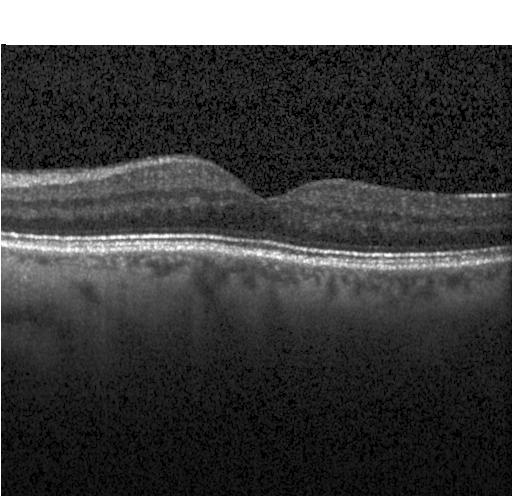 OCT scan showing neither CNV, DME, nor drusen.